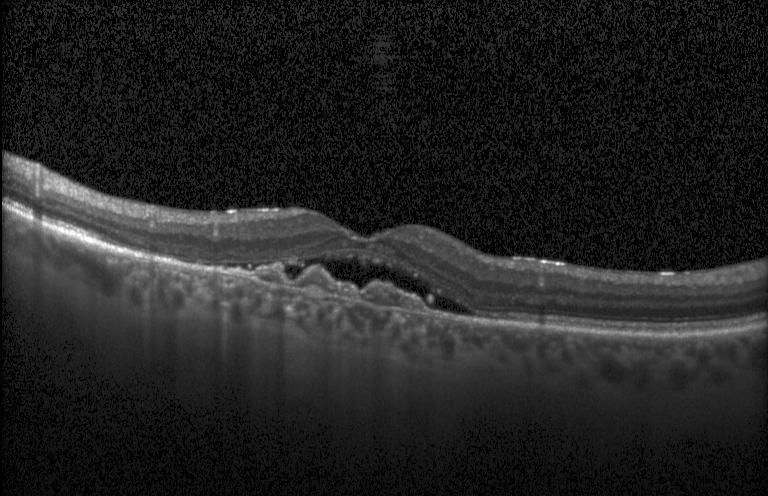
OCT scan showing CNV.